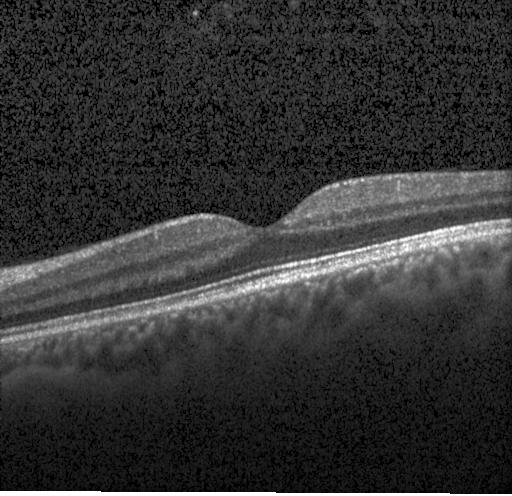 Diagnosis: no choroidal neovascularization, no diabetic macular edema, and no drusen.